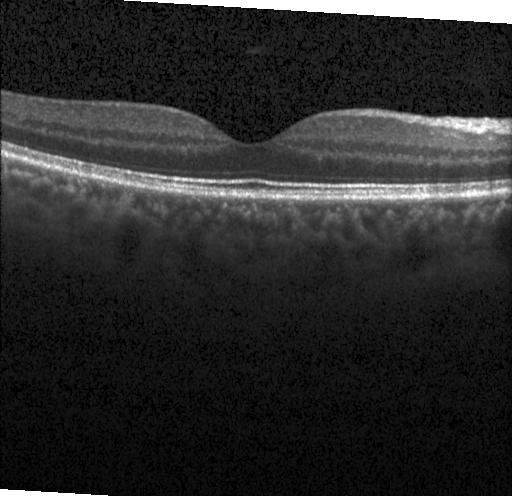 Centered on the fovea; spectral-domain OCT; retinal OCT cross-section — Finding: no evidence of choroidal neovascularization, diabetic macular edema, or drusen.